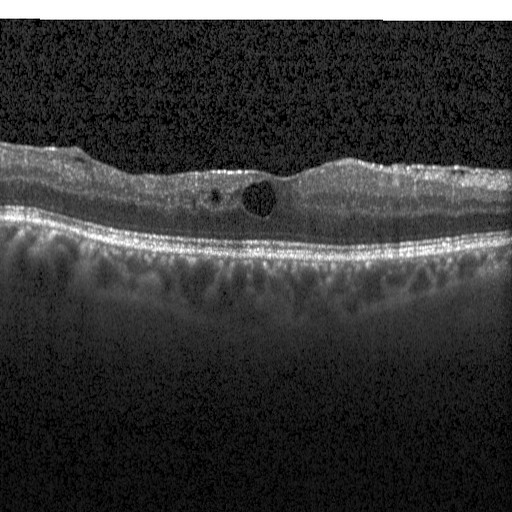 Spectral-domain optical coherence tomography. OCT B-scan. Heidelberg Spectralis OCT system. Macular OCT: diabetic macular edema.